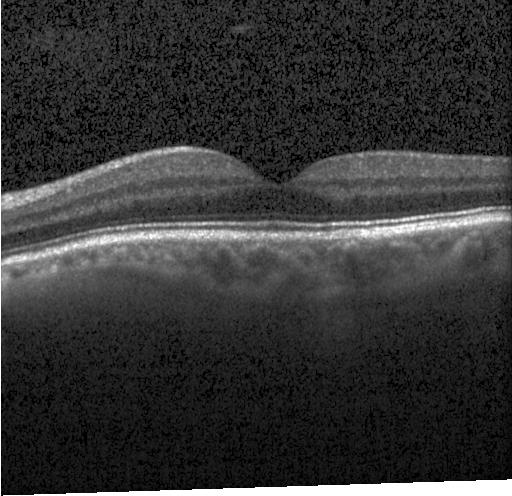
OCT B-scan; Heidelberg Spectralis OCT system. Impression: no evidence of choroidal neovascularization, diabetic macular edema, or drusen.